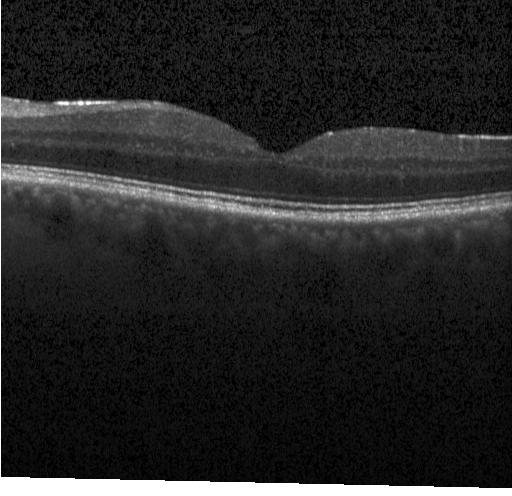

OCT finding: no choroidal neovascularization, diabetic macular edema, or drusen.